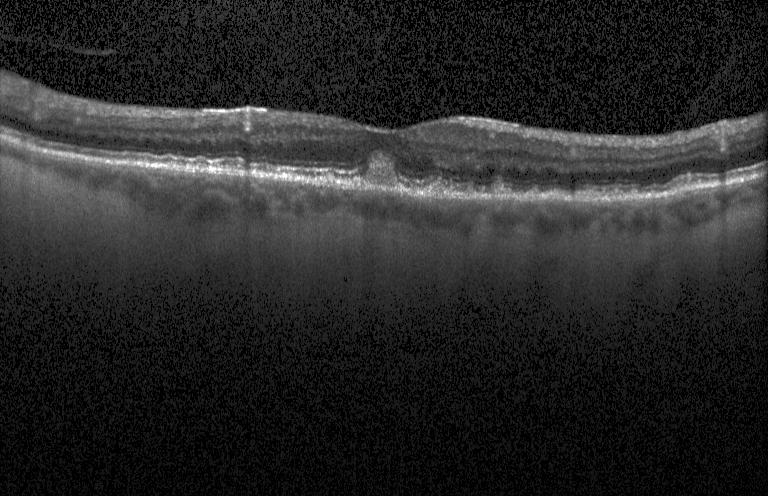 OCT line scan — Diagnosis: sub-RPE drusenoid deposits.